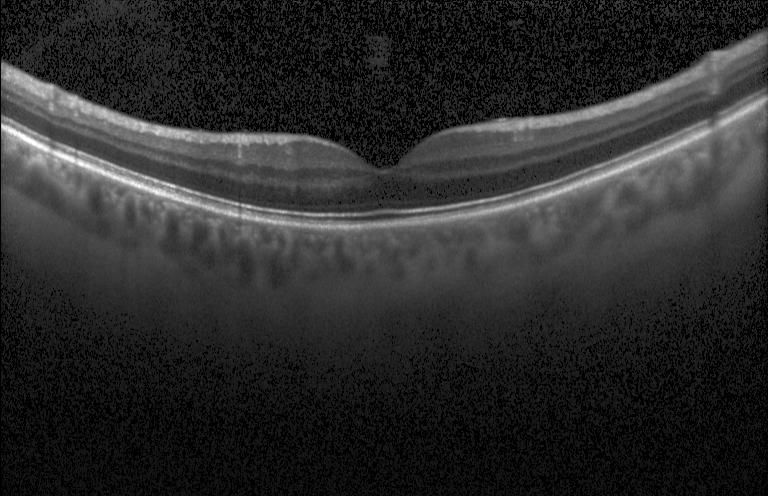
Optical coherence tomography B-scan, centered on the fovea, Heidelberg Spectralis OCT system — The scan shows neither CNV, DME, nor drusen.